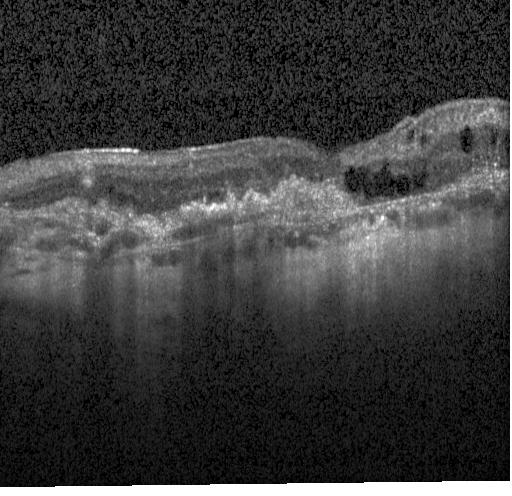
OCT line scan.
Choroidal neovascularization.